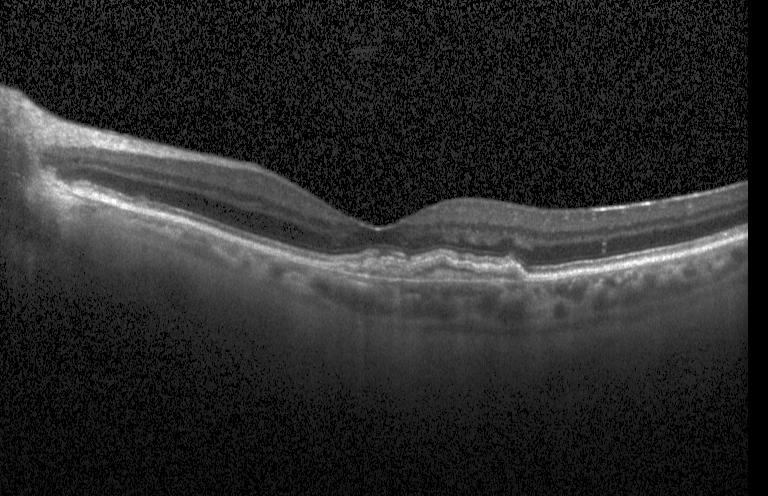

Impression: CNV.